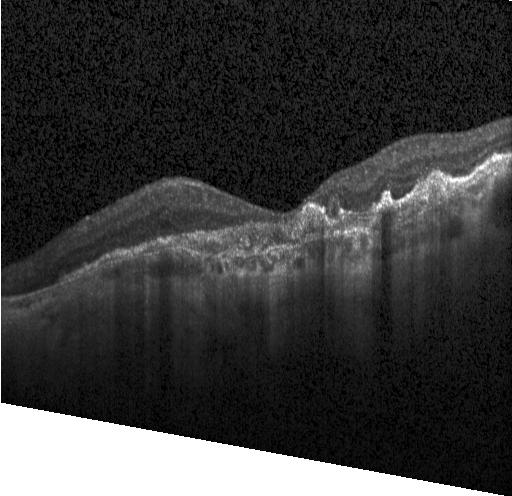
Impression: a choroidal neovascular membrane.